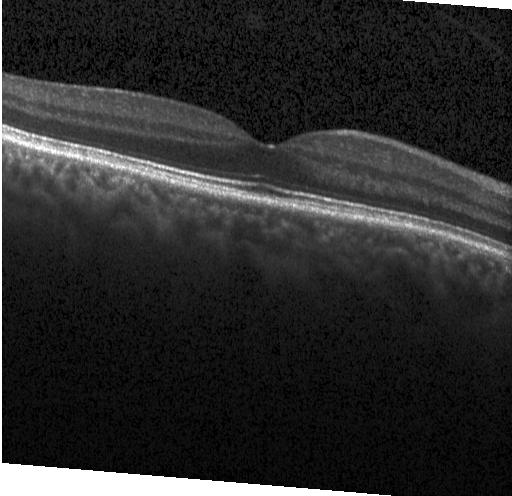
Fovea-centered, OCT line scan.
Assessment: neither choroidal neovascularization, diabetic macular edema, nor drusen.